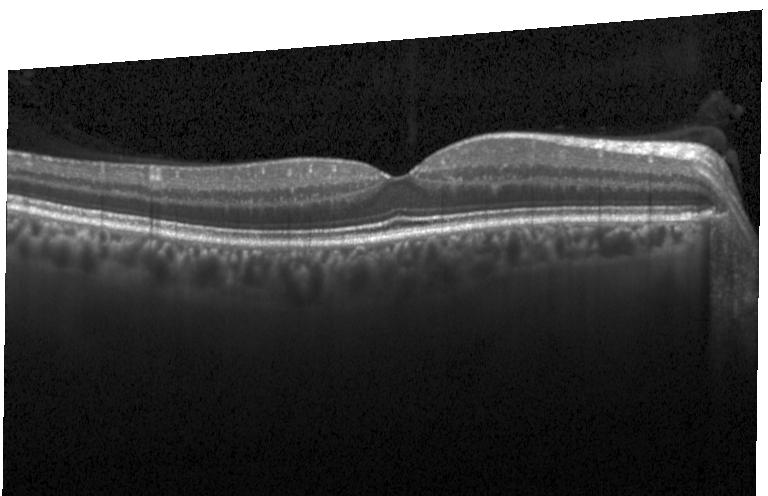

Macular OCT: neither choroidal neovascularization, diabetic macular edema, nor drusen.